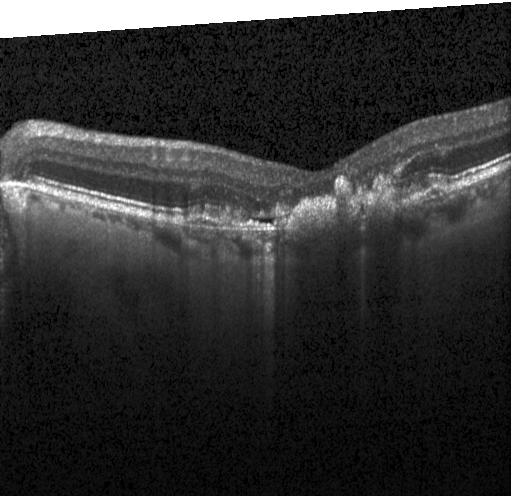
Spectral-domain OCT; OCT B-scan — Diagnosis: choroidal neovascularization.